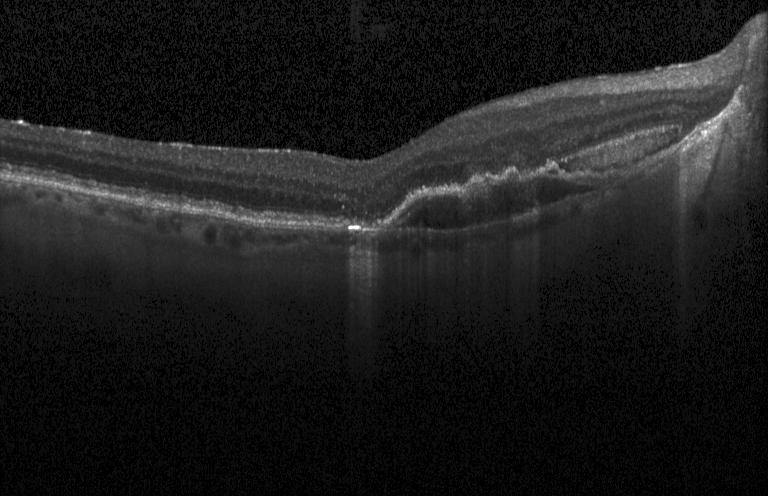 Macular OCT: a choroidal neovascular membrane.